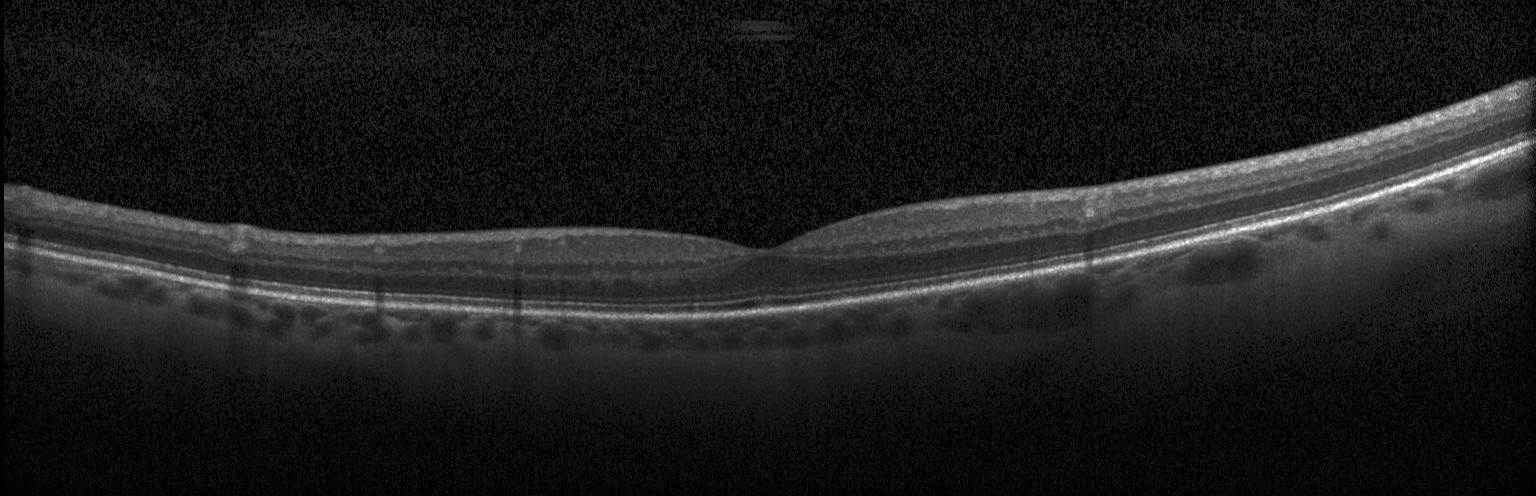

Macular OCT demonstrating no CNV, DME, or drusen.